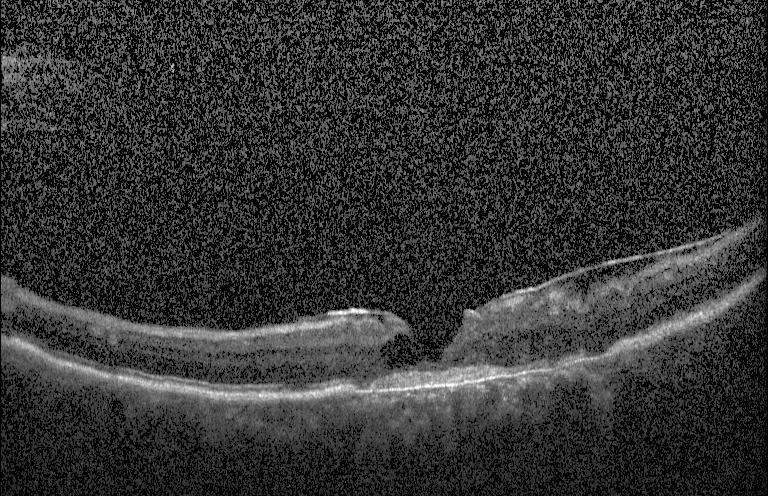
Optical coherence tomography B-scan. Centered on the fovea. Spectral-domain optical coherence tomography. Instrument: Heidelberg Spectralis
The scan shows a choroidal neovascular membrane.